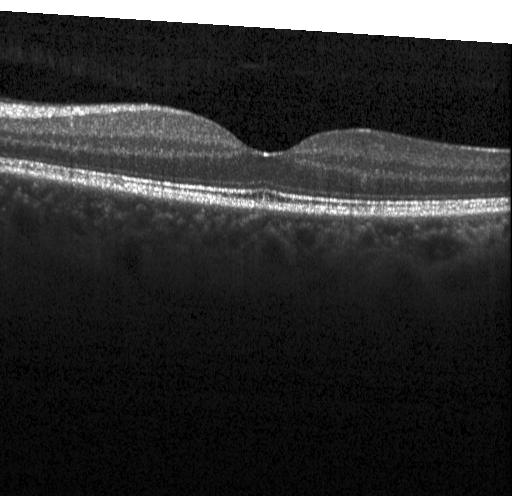

Finding: neither choroidal neovascularization, diabetic macular edema, nor drusen.